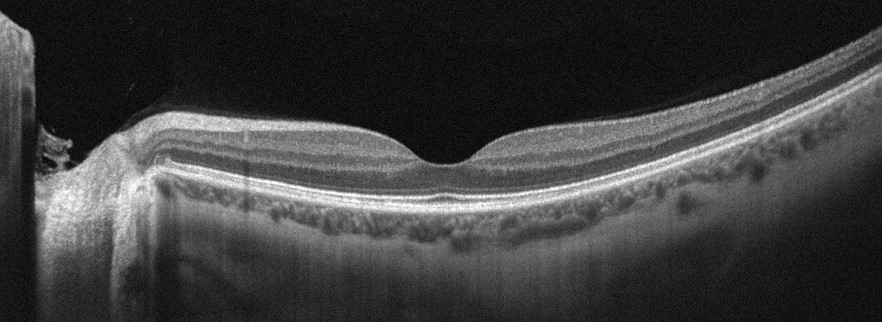
Instrument: Optovue Avanti RTVue XR, retinal OCT cross-section. OCT finding: no evidence of AMD, DME, ERM, RAO, RVO, or VID.